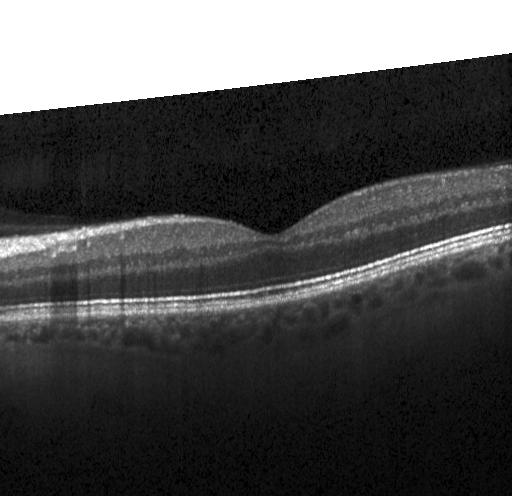 Finding: neither CNV, DME, nor drusen.